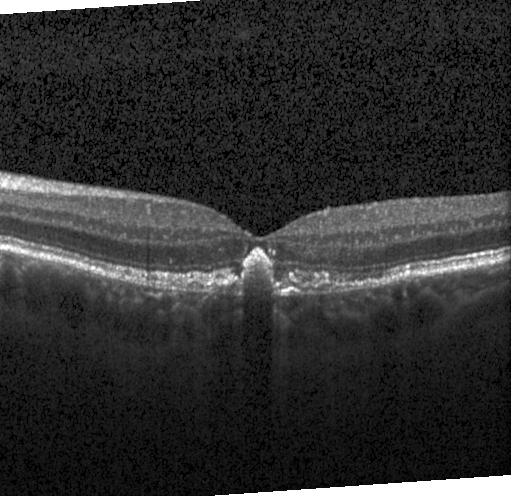
OCT B-scan.
Impression: CNV.